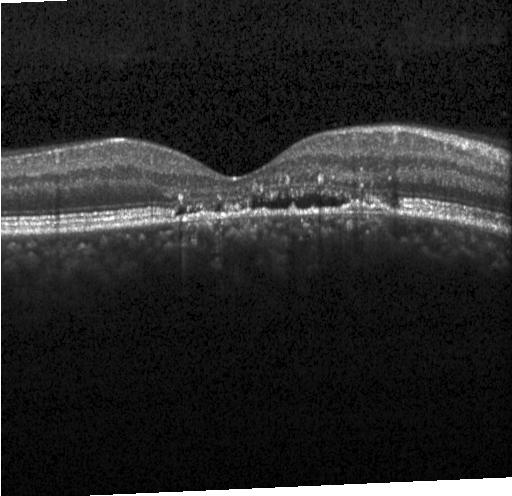 This B-scan demonstrates a choroidal neovascular membrane.